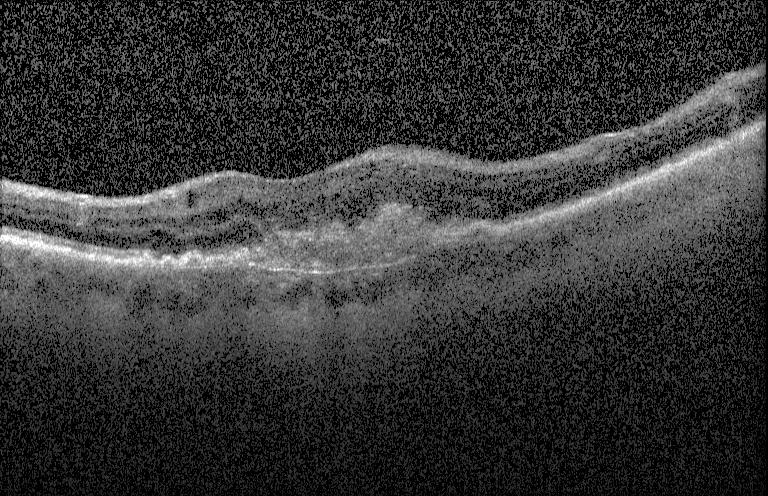 Instrument: Heidelberg Spectralis. OCT B-scan
Assessment: CNV.